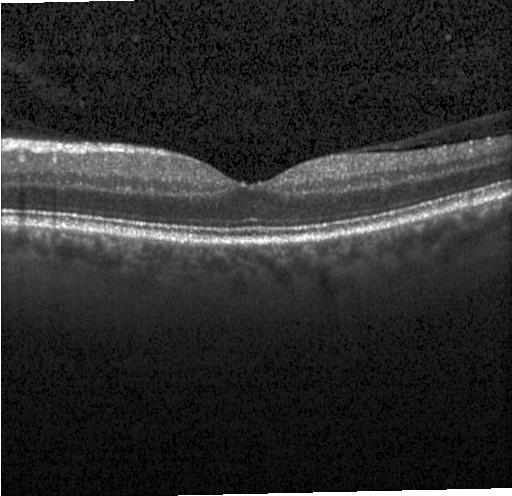

OCT B-scan
Impression: neither CNV, DME, nor drusen.